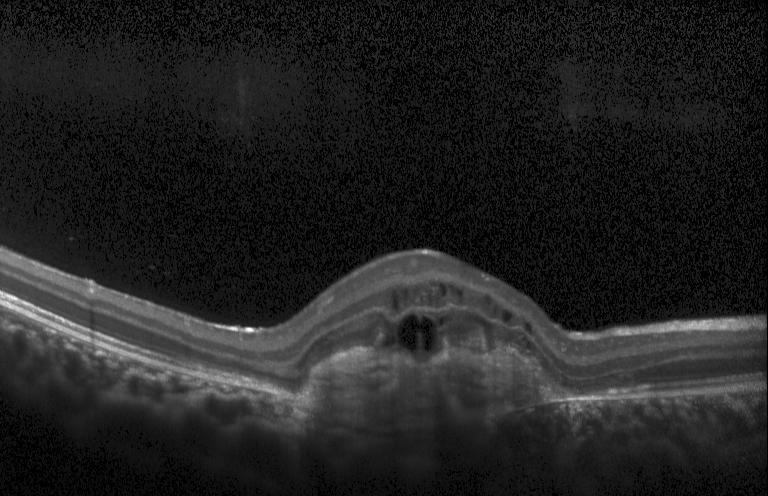 This B-scan demonstrates choroidal neovascularization.